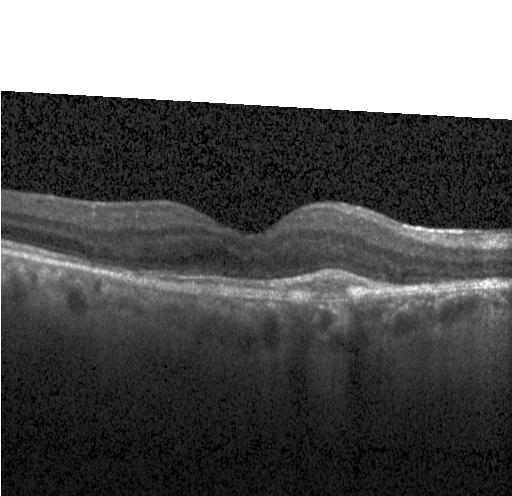

Through the macula, spectral-domain optical coherence tomography, optical coherence tomography scan. Finding: choroidal neovascularization (CNV).